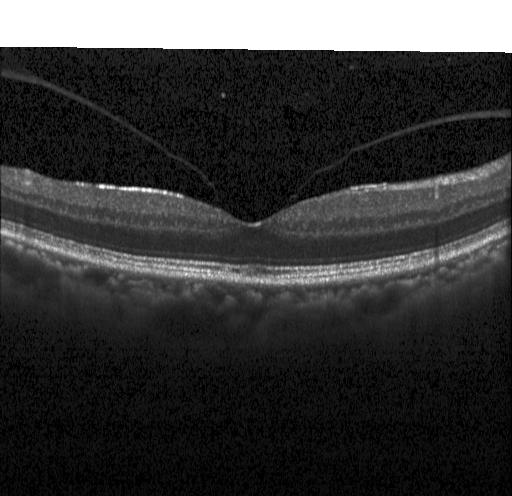 Optical coherence tomography B-scan · Heidelberg Spectralis. Impression: no evidence of choroidal neovascularization, diabetic macular edema, or drusen.